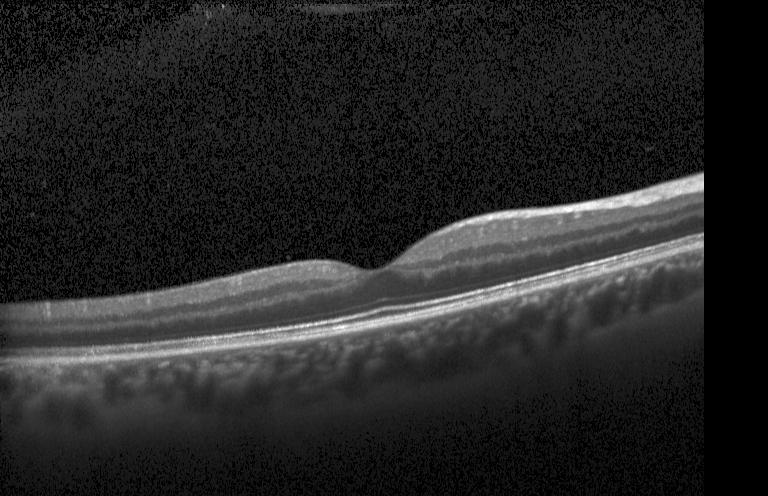 Optical coherence tomography scan
Diagnosis: no evidence of choroidal neovascularization, diabetic macular edema, or drusen.